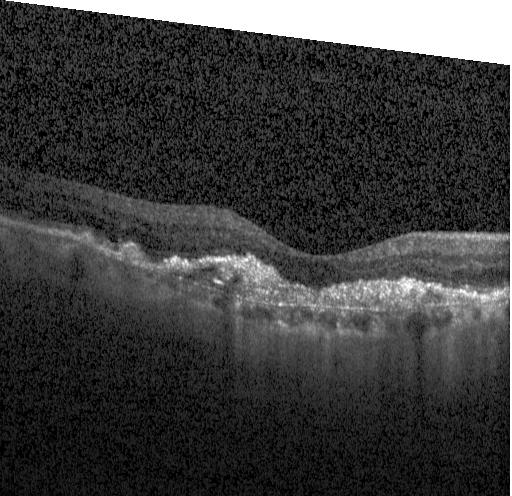

Through the macula; OCT B-scan; spectral-domain optical coherence tomography; Heidelberg Spectralis OCT system. Impression: a choroidal neovascular membrane.